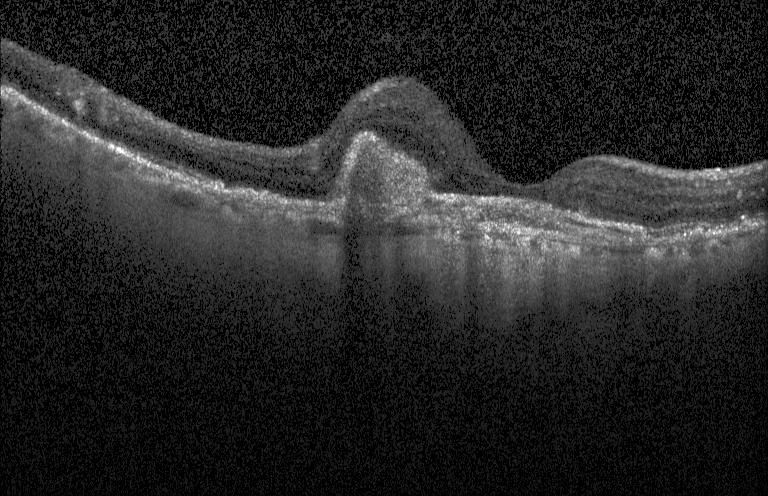

OCT line scan; centered on the fovea.
Diagnosis: choroidal neovascularization.